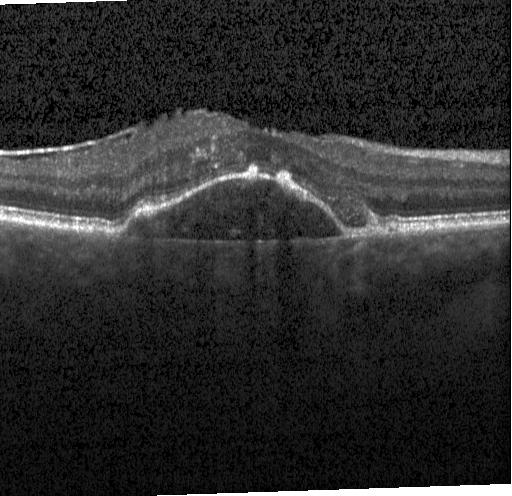 Spectral-domain optical coherence tomography · macular scan · optical coherence tomography scan — Diagnosis: a choroidal neovascular membrane.